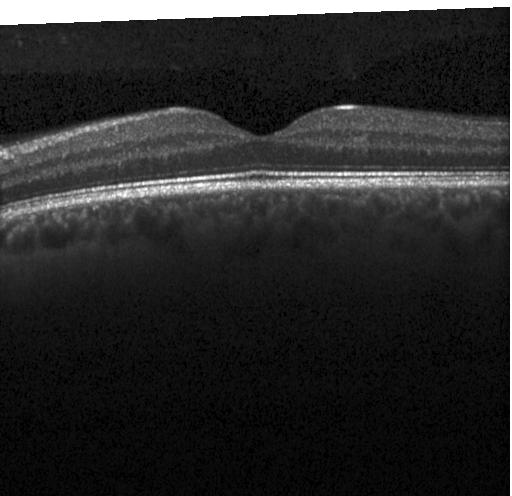
Acquired on a Heidelberg Spectralis, spectral-domain OCT, optical coherence tomography B-scan.
Dx: no evidence of CNV, DME, or drusen.